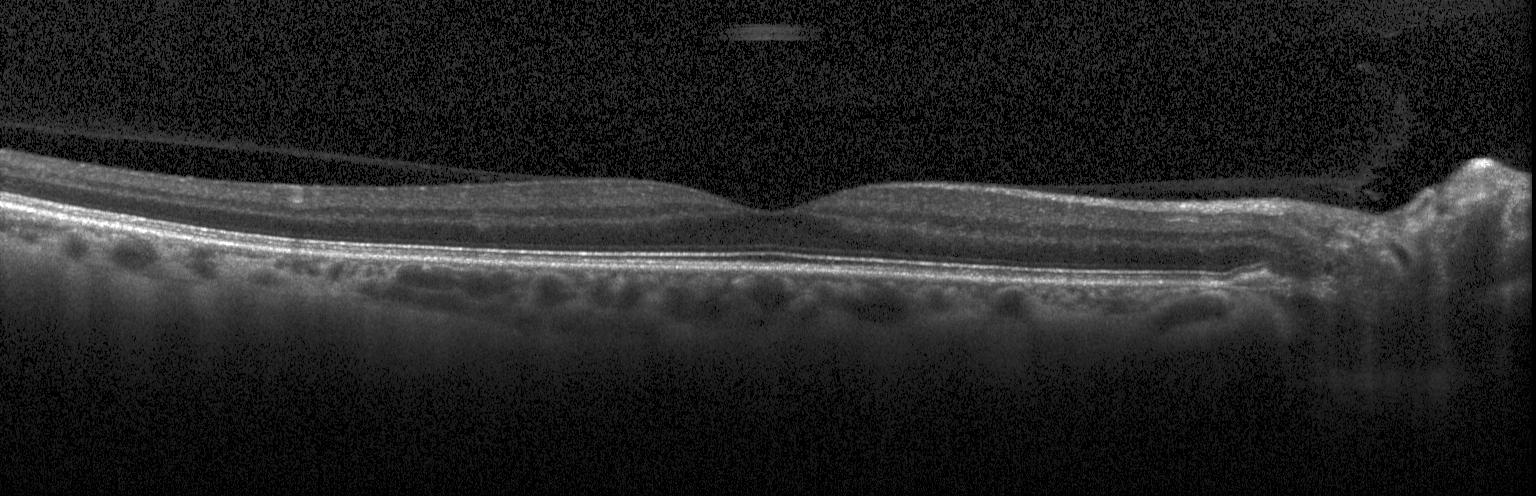 Fovea-centered; retinal OCT cross-section; instrument: Heidelberg Spectralis; SD-OCT. Finding: no choroidal neovascularization, diabetic macular edema, or drusen.